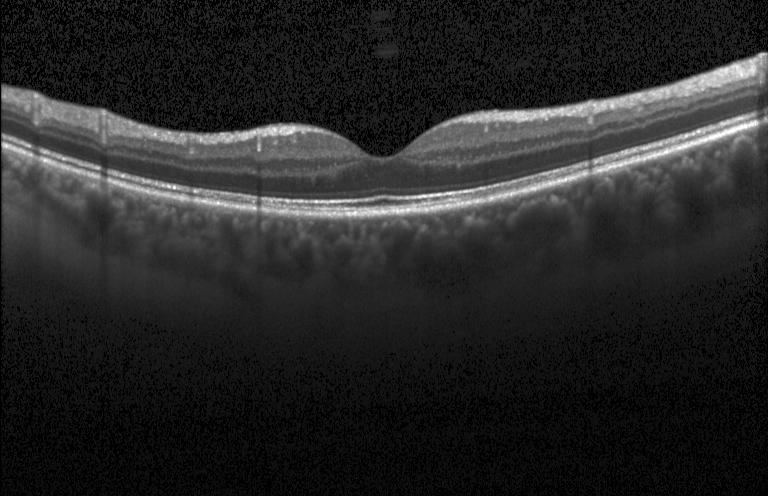 Centered on the fovea · Heidelberg Spectralis OCT system · retinal OCT cross-section.
This B-scan demonstrates neither choroidal neovascularization, diabetic macular edema, nor drusen.